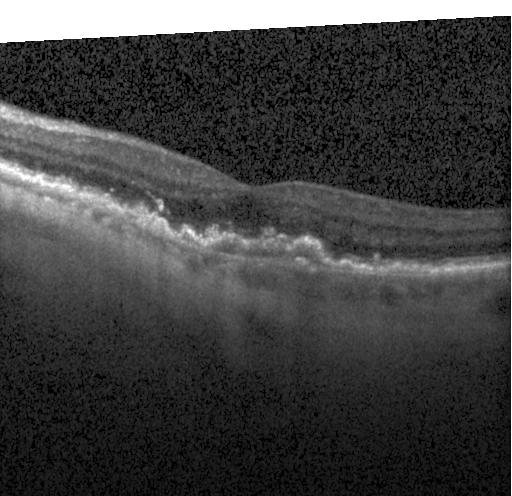 OCT line scan
This B-scan demonstrates a choroidal neovascular membrane.